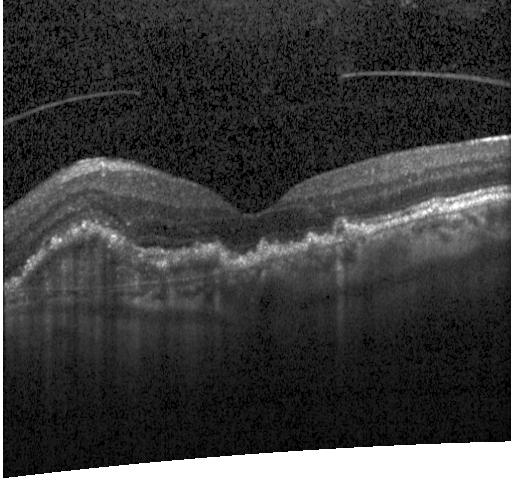
Finding: a choroidal neovascular membrane.